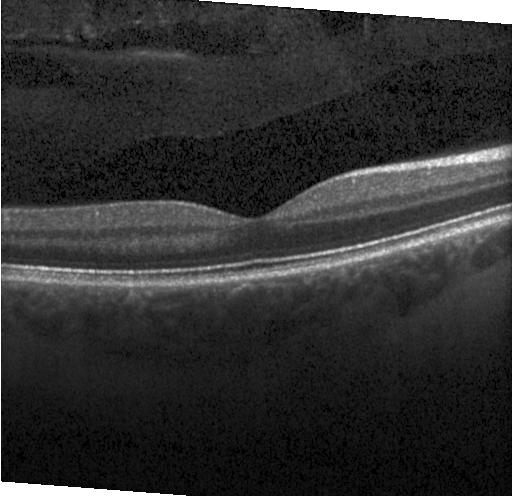
Heidelberg Spectralis OCT system, fovea-centered, SD-OCT, retinal OCT cross-section. No evidence of CNV, DME, or drusen.